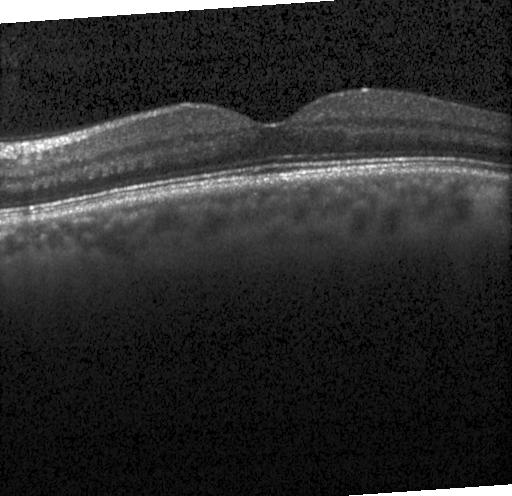 Optical coherence tomography B-scan, Heidelberg Spectralis, SD-OCT. Finding: no choroidal neovascularization, diabetic macular edema, or drusen.